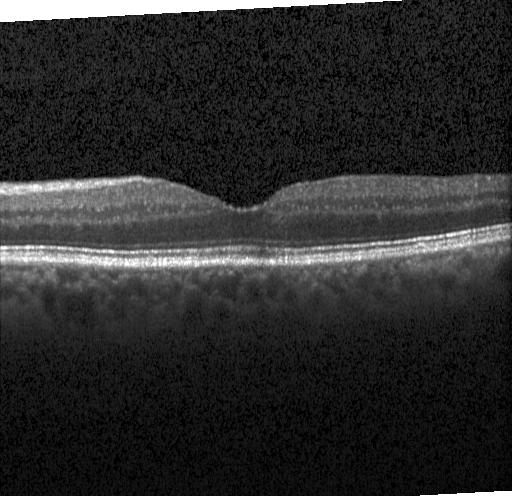
OCT B-scan. Finding: no evidence of CNV, DME, or drusen.